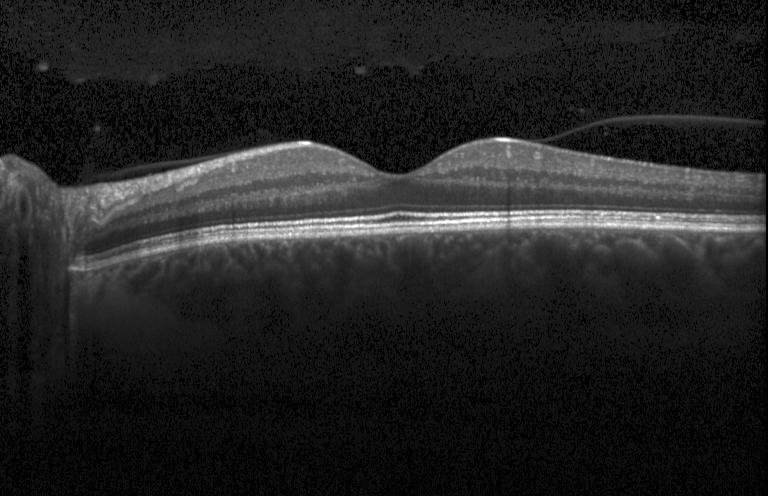
Impression: no choroidal neovascularization, no diabetic macular edema, and no drusen.